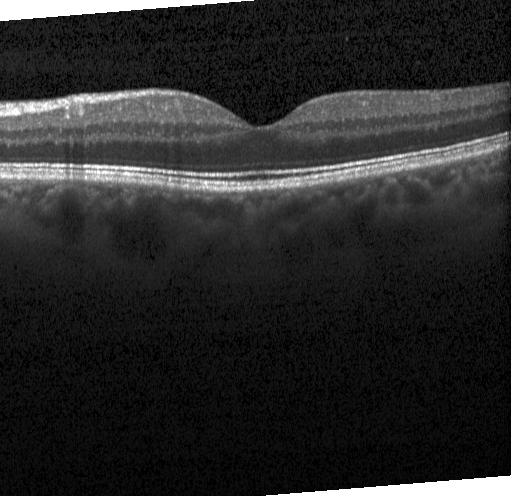
Spectral-domain OCT B-scan: no choroidal neovascularization, diabetic macular edema, or drusen.